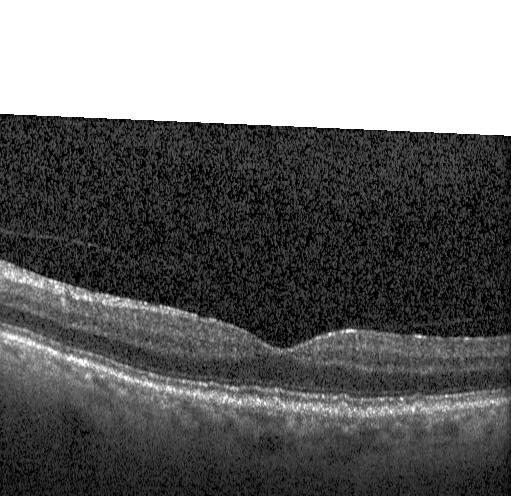
Retinal OCT cross-section — Impression: drusen.